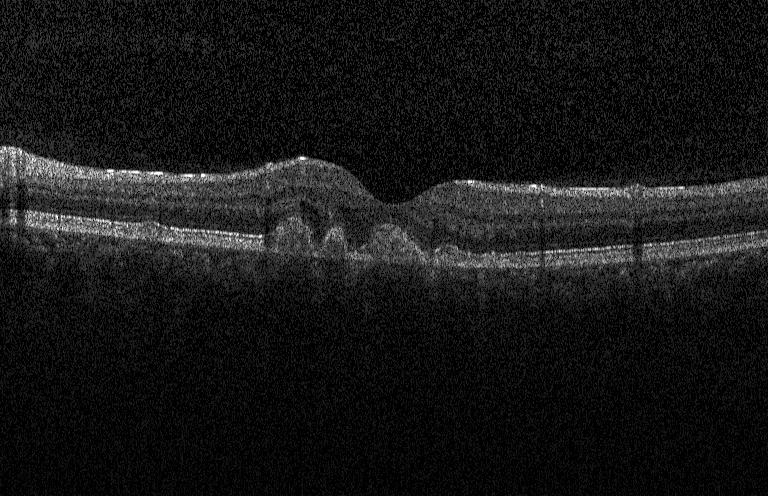 Fovea-centered; SD-OCT; instrument: Heidelberg Spectralis; retinal OCT B-scan.
Impression: drusen.